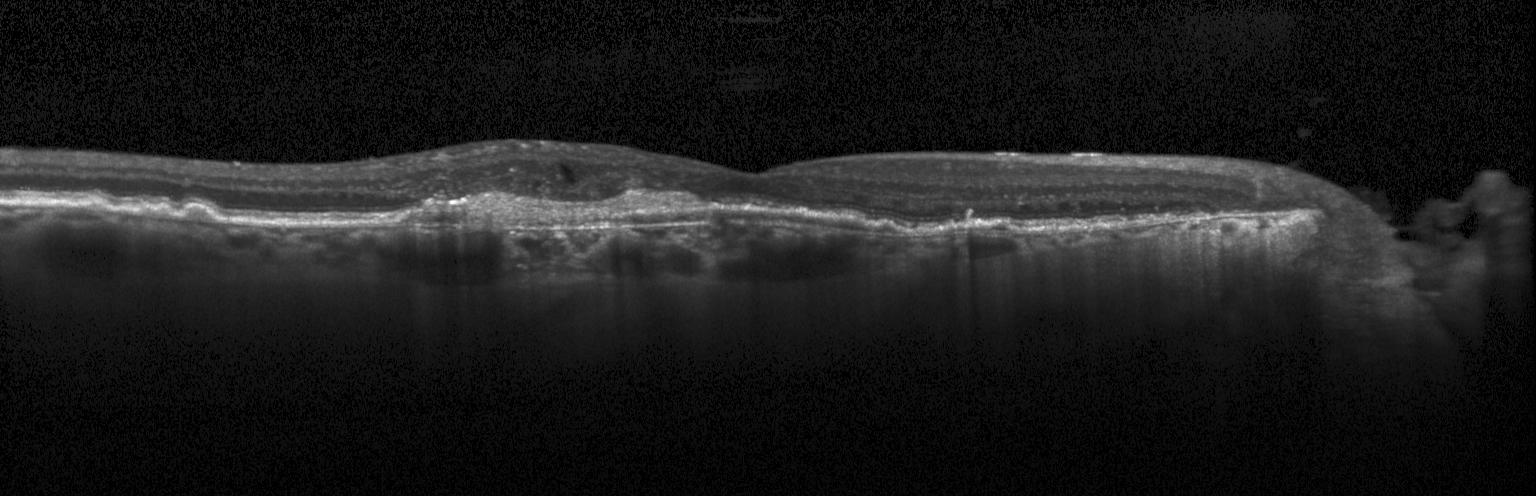 Impression: choroidal neovascularization (CNV).